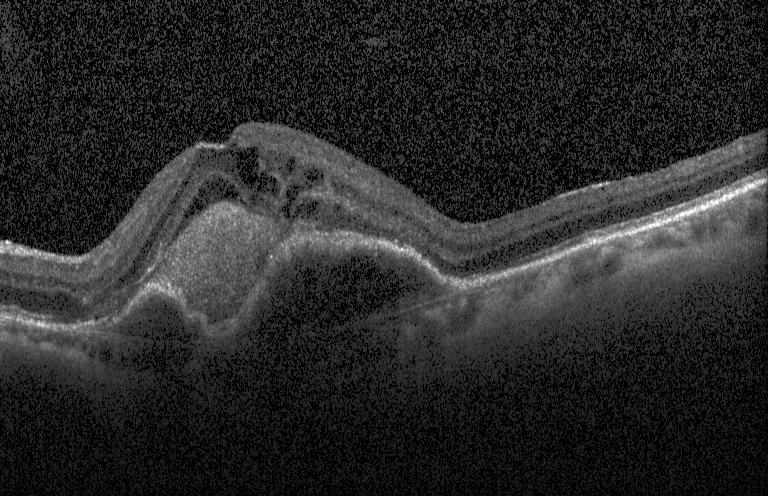
Finding: a choroidal neovascular membrane.